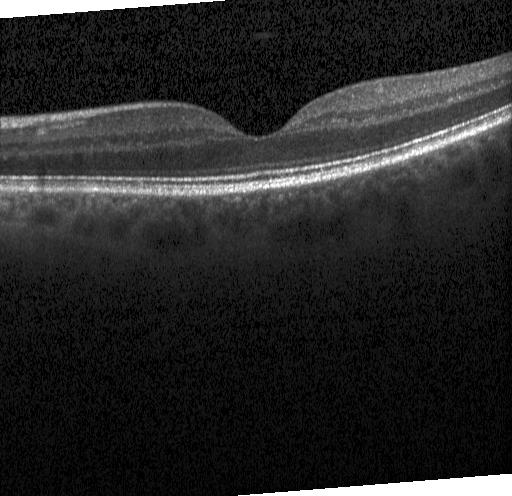

Finding: no choroidal neovascularization, no diabetic macular edema, and no drusen.